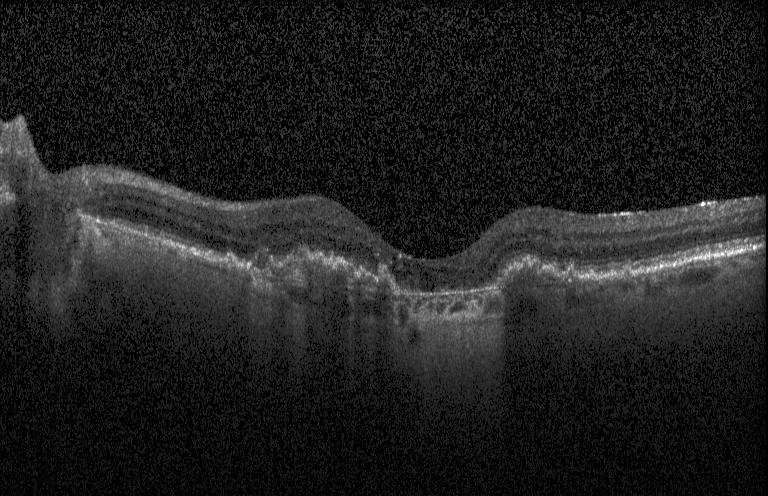
Retinal OCT B-scan
Impression: a choroidal neovascular membrane.